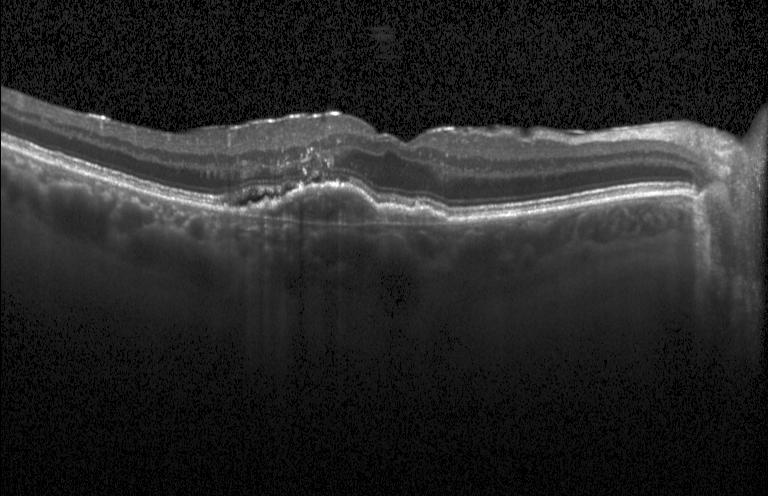
OCT line scan.
Macular OCT: CNV.